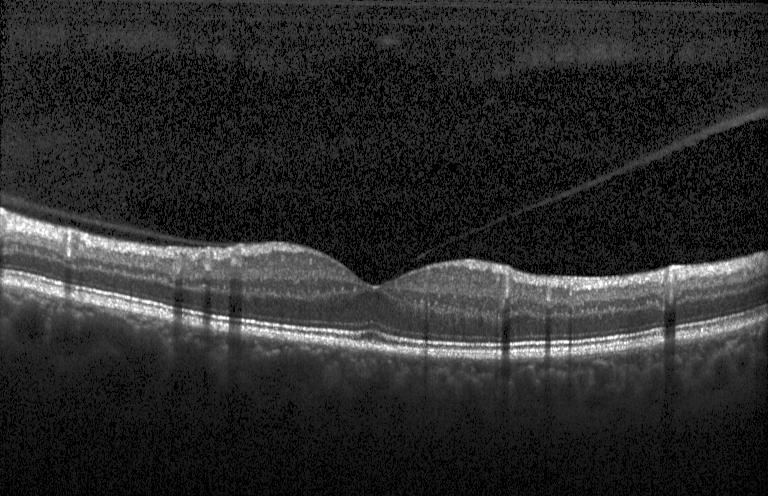
This B-scan demonstrates no evidence of CNV, DME, or drusen.